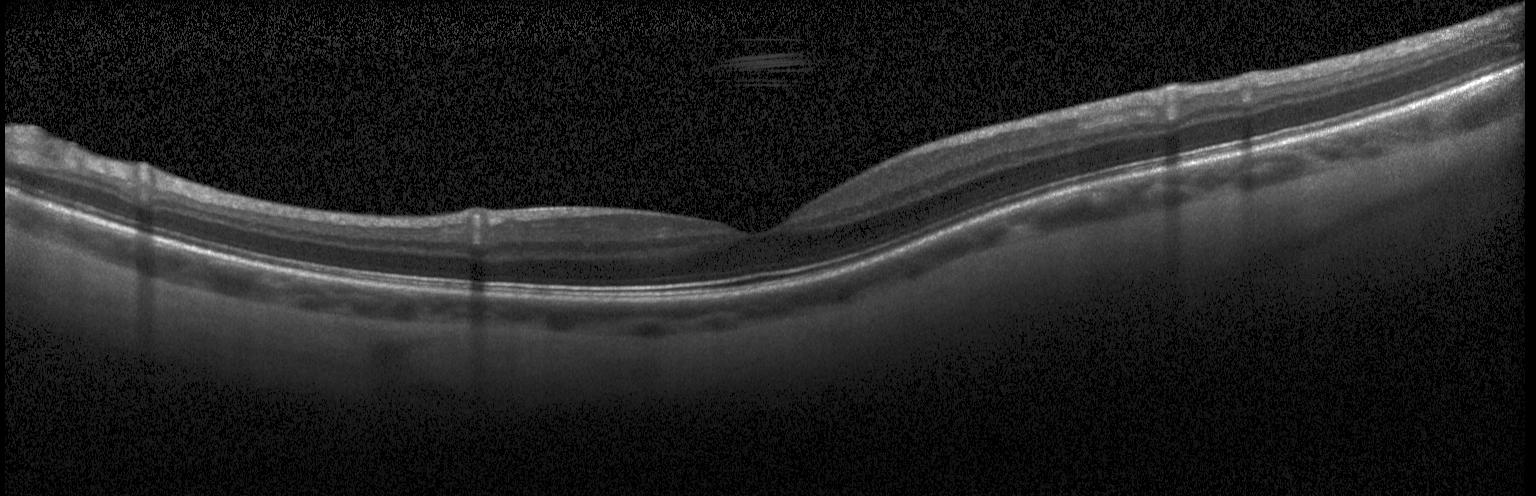 The scan shows no evidence of choroidal neovascularization, diabetic macular edema, or drusen.